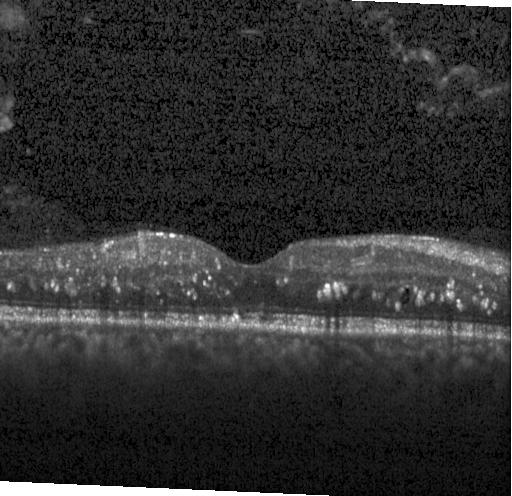

The scan shows DME.